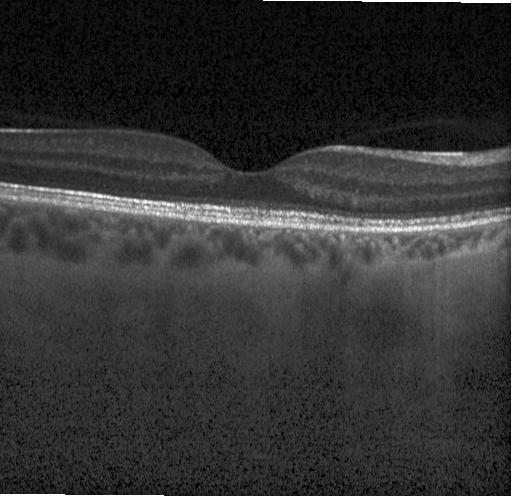 OCT line scan. Dx: no choroidal neovascularization, diabetic macular edema, or drusen.